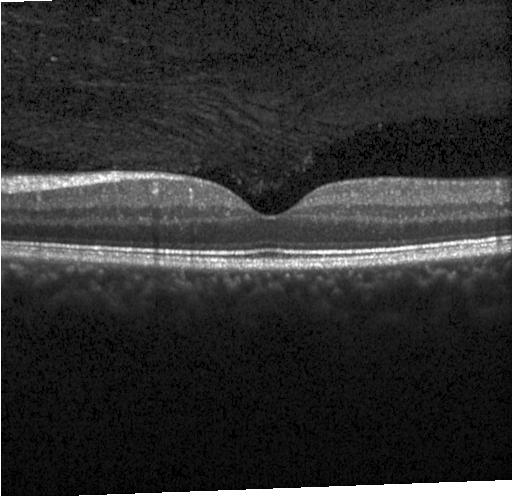

Retinal OCT cross-section; Heidelberg Spectralis OCT system — Assessment: no choroidal neovascularization, diabetic macular edema, or drusen.